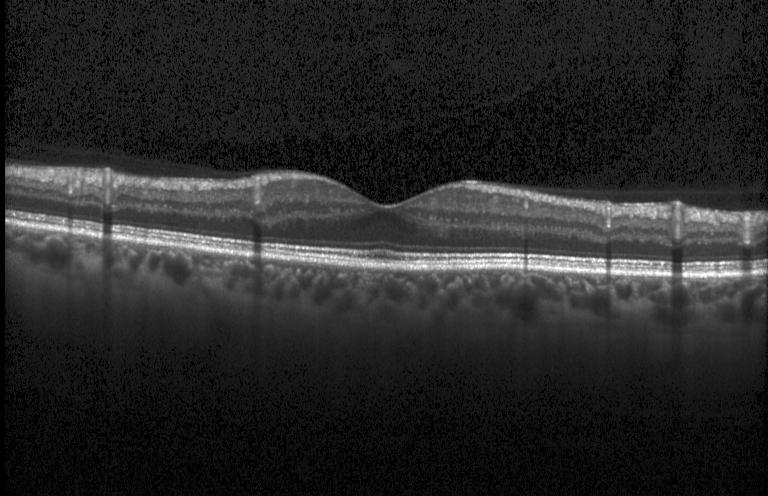
OCT scan showing neither CNV, DME, nor drusen.